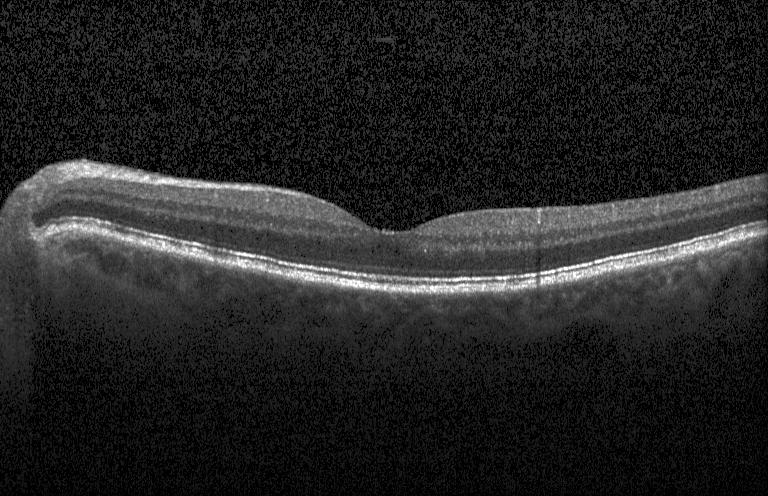 Dx: no evidence of choroidal neovascularization, diabetic macular edema, or drusen.